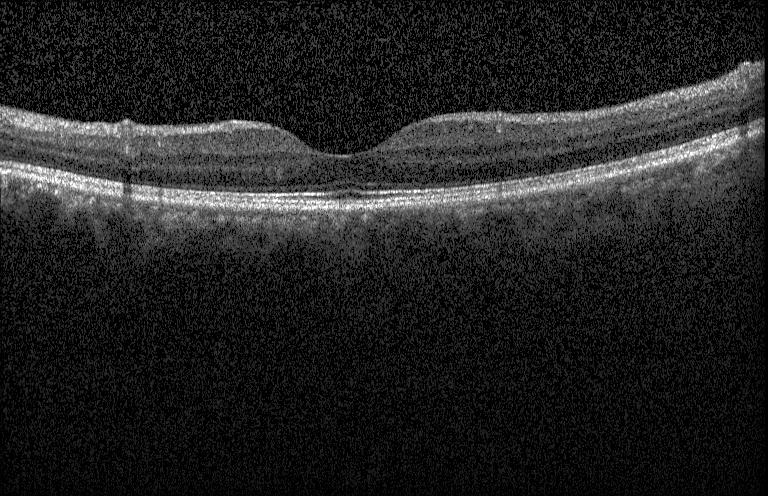 Spectral-domain optical coherence tomography; retinal OCT cross-section; Heidelberg Spectralis OCT system; macular scan
Diagnosis: no evidence of choroidal neovascularization, diabetic macular edema, or drusen.